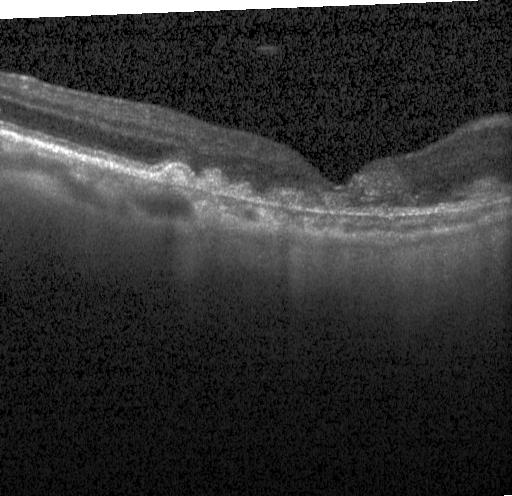

Optical coherence tomography scan — OCT finding: CNV.